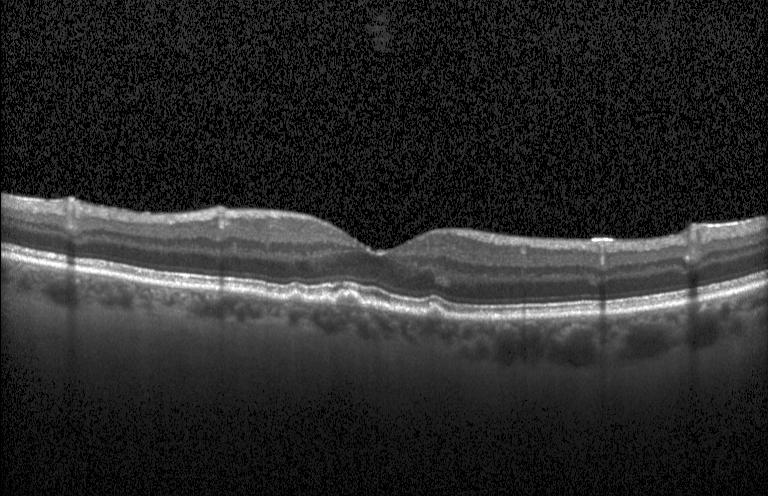

Diagnosis: drusen.